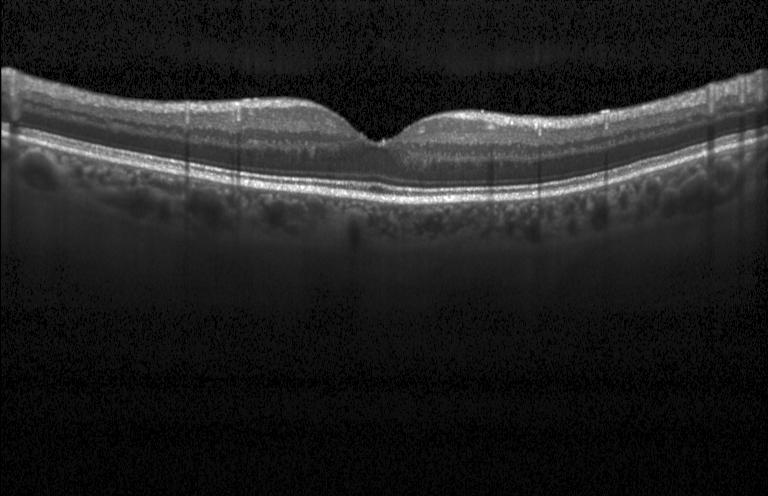 Spectral-domain optical coherence tomography; retinal OCT cross-section; through the macula; acquired on a Heidelberg Spectralis.
Diagnosis: no CNV, no DME, and no drusen.